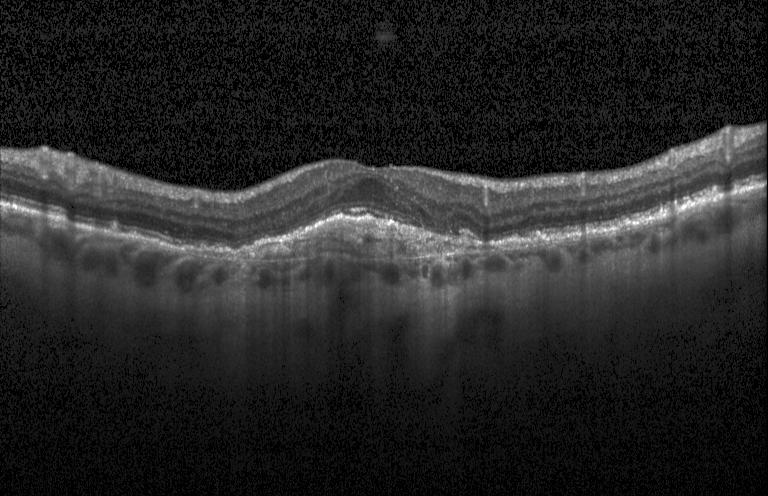

Retinal OCT B-scan.
Impression: CNV.